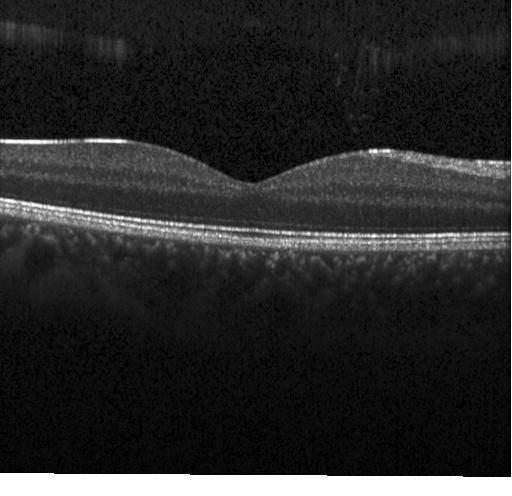

Retinal OCT cross-section showing no choroidal neovascularization, no diabetic macular edema, and no drusen.